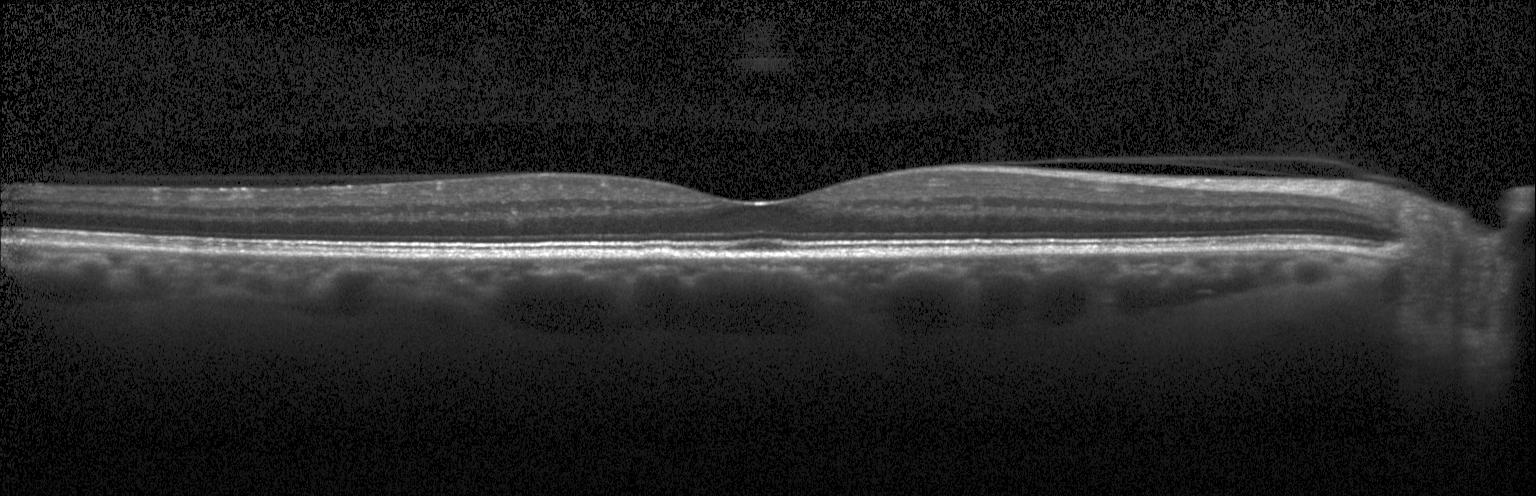
Finding: no evidence of choroidal neovascularization, diabetic macular edema, or drusen.